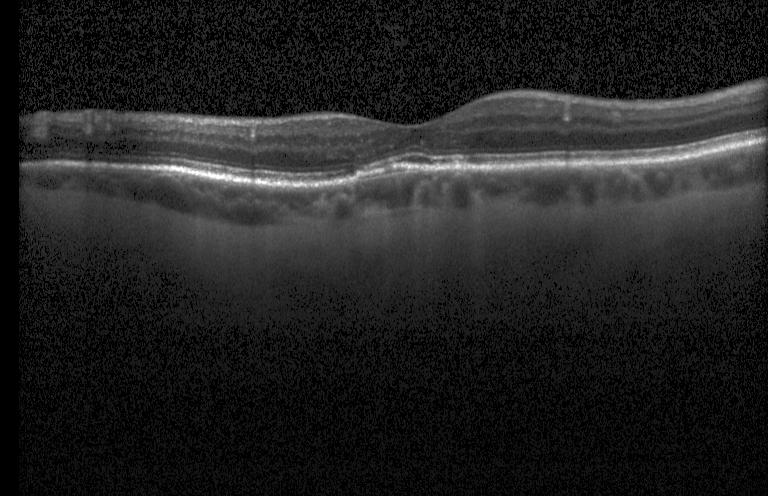 Assessment: a choroidal neovascular membrane.